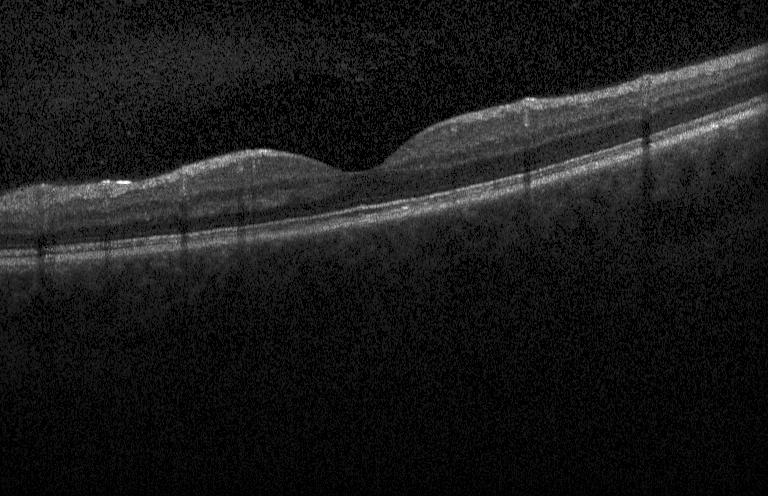

Spectral-domain optical coherence tomography; optical coherence tomography B-scan.
Assessment: no CNV, no DME, and no drusen.